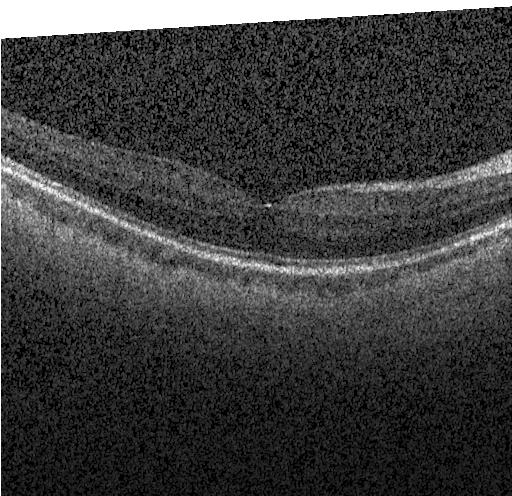 Acquired on a Heidelberg Spectralis · spectral-domain optical coherence tomography · OCT B-scan · centered on the fovea — Impression: no choroidal neovascularization, no diabetic macular edema, and no drusen.